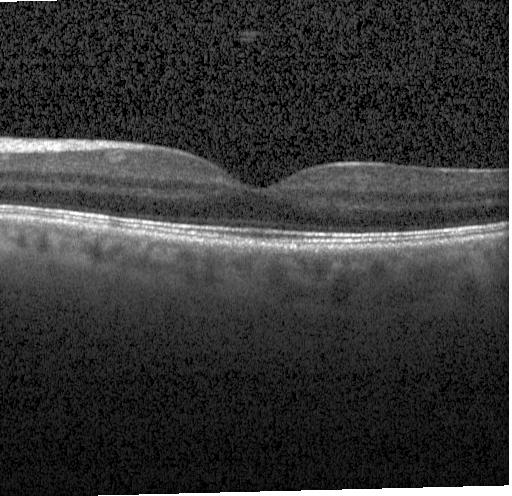 No evidence of choroidal neovascularization, diabetic macular edema, or drusen.